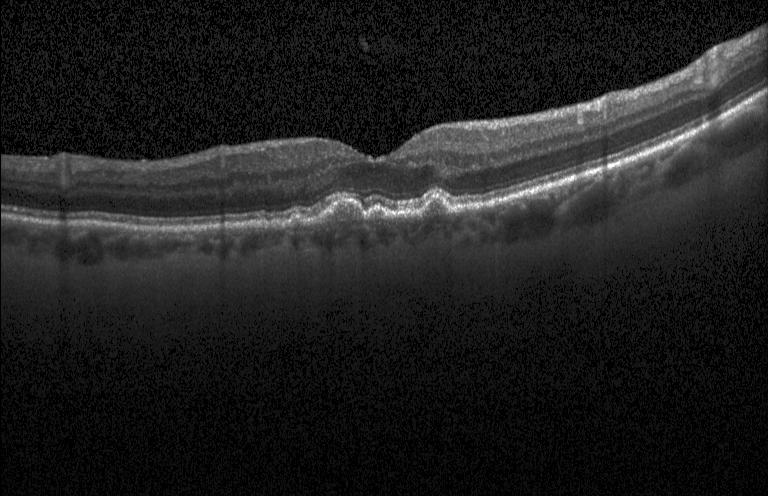
OCT B-scan; centered on the fovea; Heidelberg Spectralis OCT system — Impression: multiple drusen.